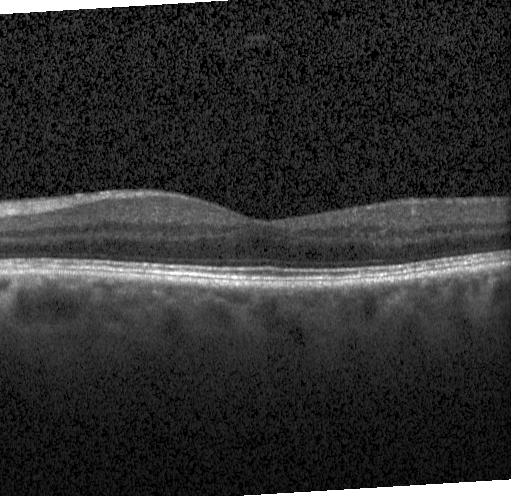
Diagnosis: no choroidal neovascularization, no diabetic macular edema, and no drusen.